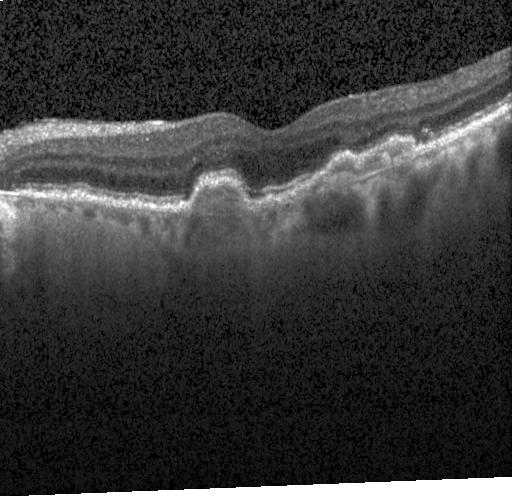 Through the macula, Heidelberg Spectralis OCT system, SD-OCT, retinal OCT B-scan
CNV.